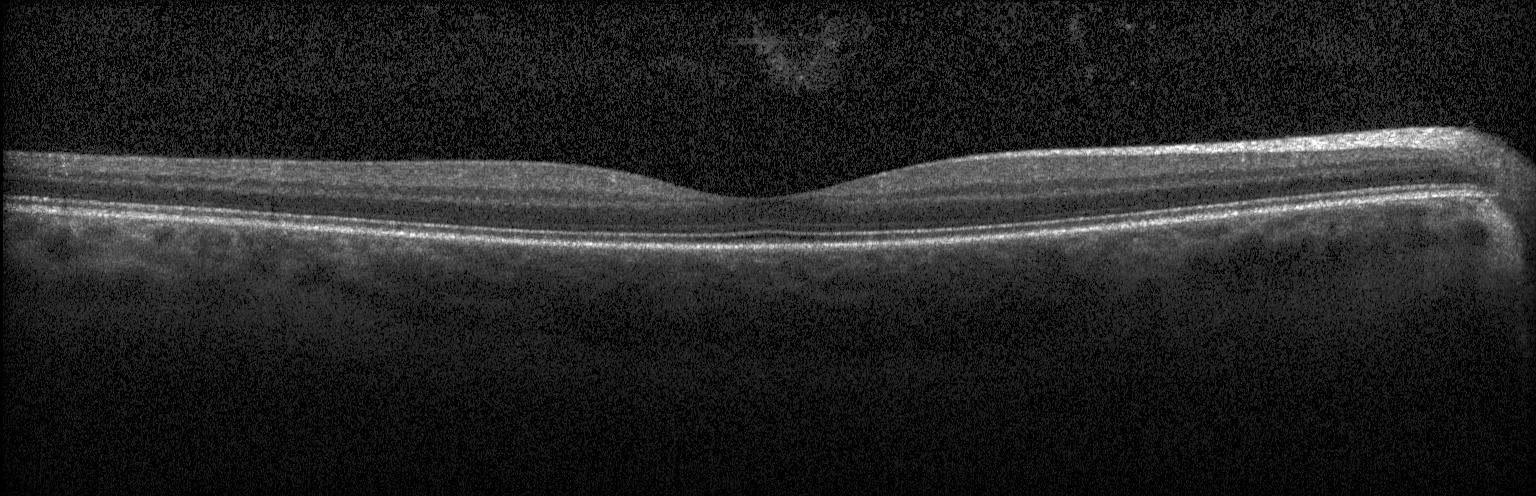

OCT B-scan. Instrument: Heidelberg Spectralis.
OCT finding: no evidence of CNV, DME, or drusen.